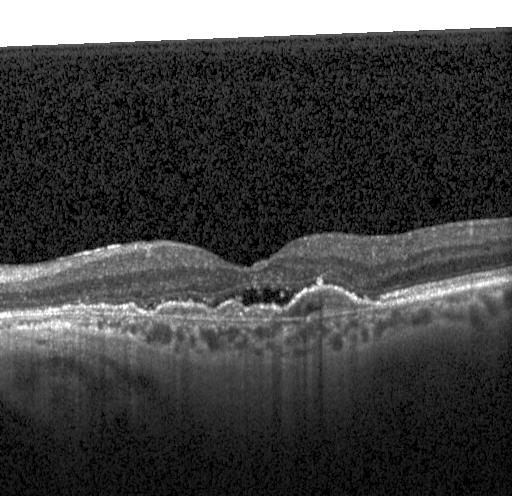 SD-OCT. Through the macula. Retinal OCT B-scan
The scan shows choroidal neovascularization.